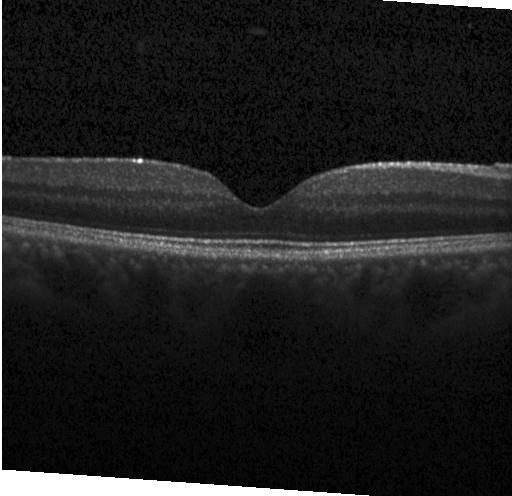

Diagnosis: neither choroidal neovascularization, diabetic macular edema, nor drusen.